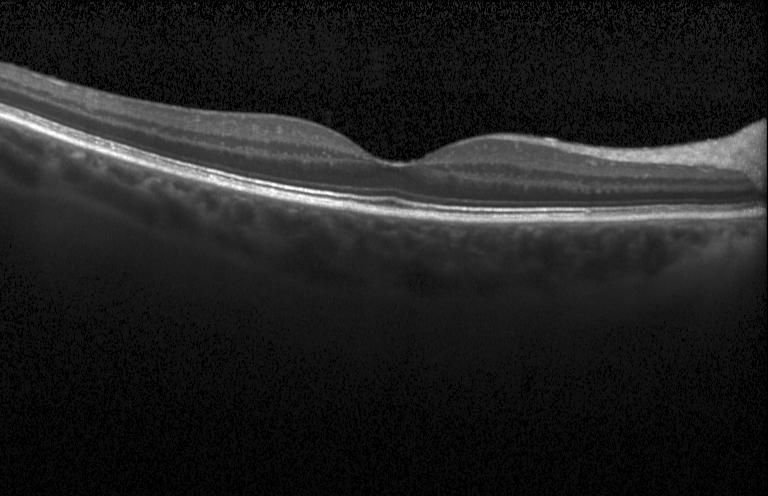
OCT line scan · acquired on a Heidelberg Spectralis · fovea-centered.
Diagnosis: no choroidal neovascularization, diabetic macular edema, or drusen.